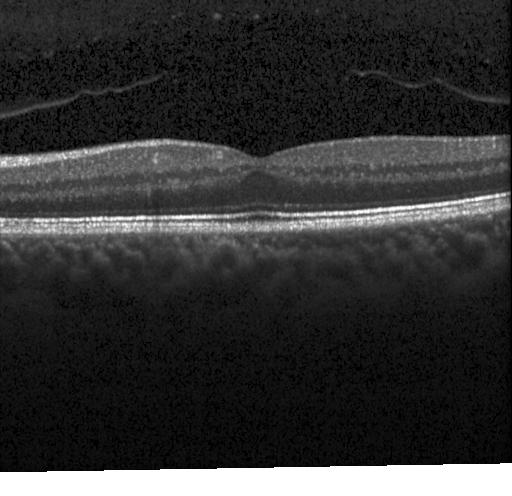 Spectral-domain OCT. Instrument: Heidelberg Spectralis. OCT B-scan. Dx: no CNV, no DME, and no drusen.